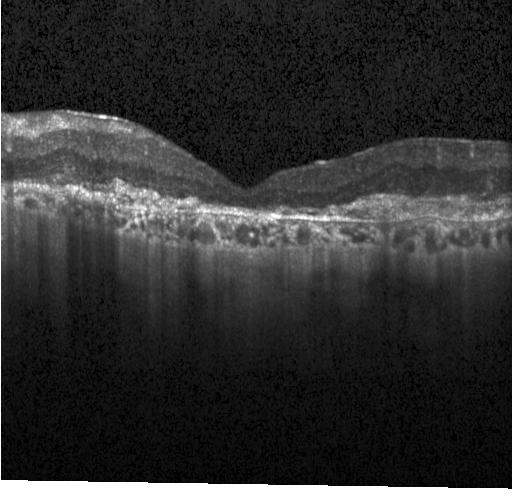

Optical coherence tomography B-scan · fovea-centered · spectral-domain OCT · instrument: Heidelberg Spectralis. This B-scan demonstrates a choroidal neovascular membrane.